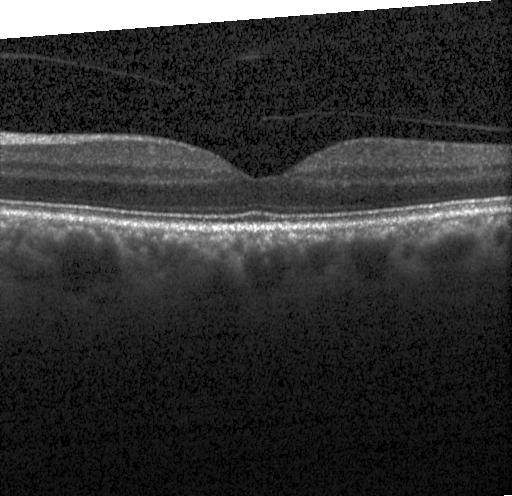 Macular OCT demonstrating no CNV, DME, or drusen.